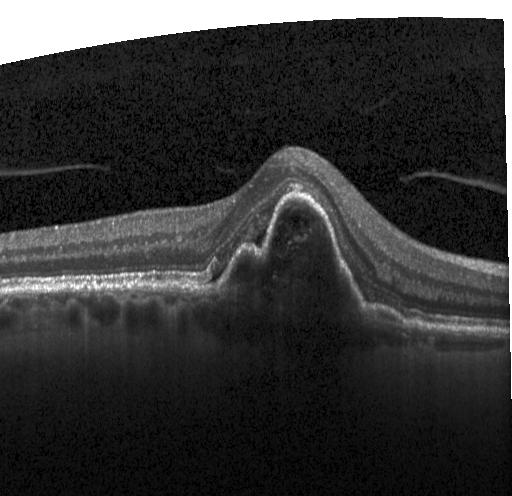

SD-OCT. Instrument: Heidelberg Spectralis. Horizontal scan through the fovea. Retinal OCT cross-section — Impression: a choroidal neovascular membrane.